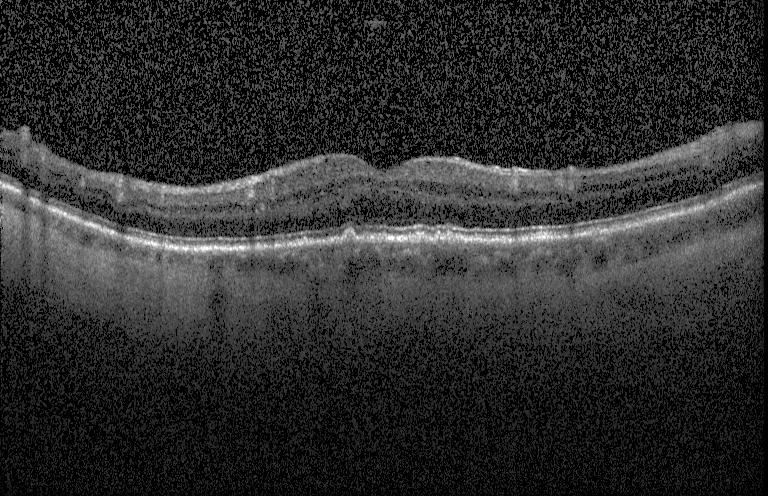
OCT scan showing sub-RPE drusenoid deposits.